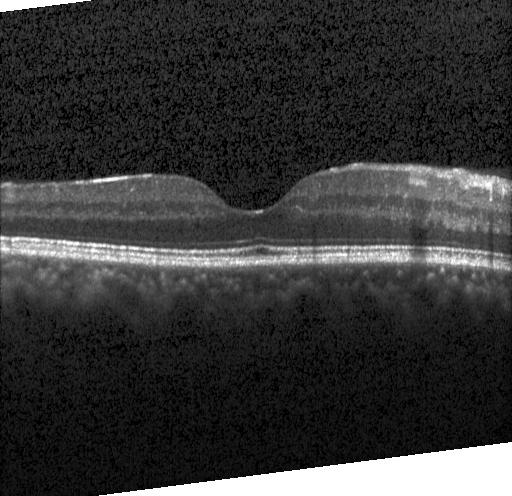

Instrument: Heidelberg Spectralis; fovea-centered; OCT B-scan. OCT finding: no CNV, DME, or drusen.